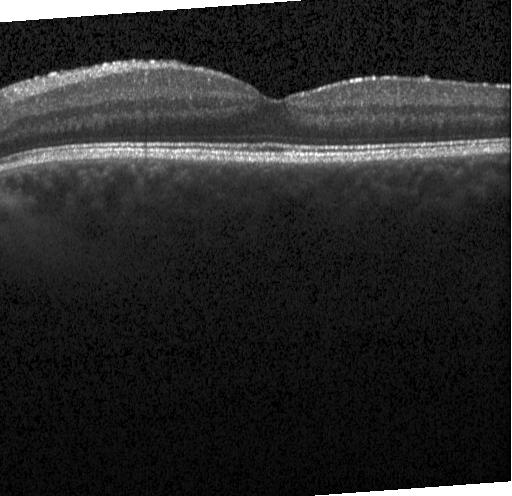

OCT B-scan · fovea-centered — Diagnosis: no choroidal neovascularization, no diabetic macular edema, and no drusen.